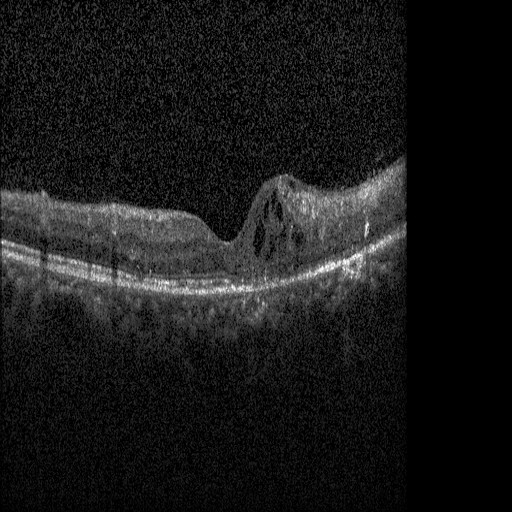

Heidelberg Spectralis OCT system · OCT B-scan.
Impression: diabetic macular edema.